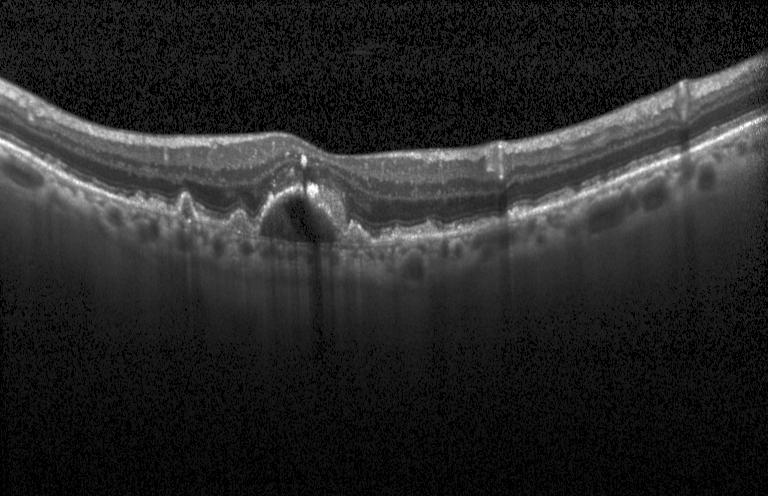
Retinal OCT cross-section.
This B-scan demonstrates CNV.